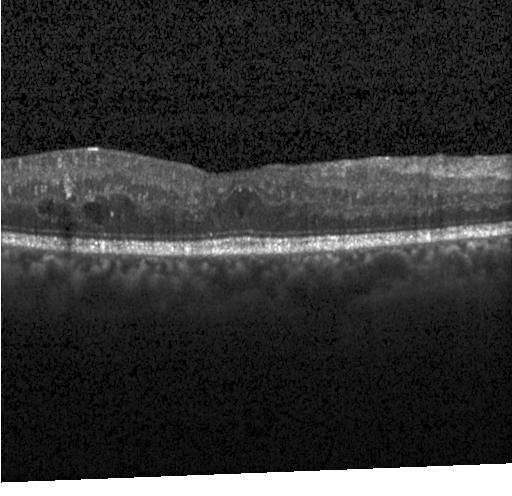 Diagnosis: DME.